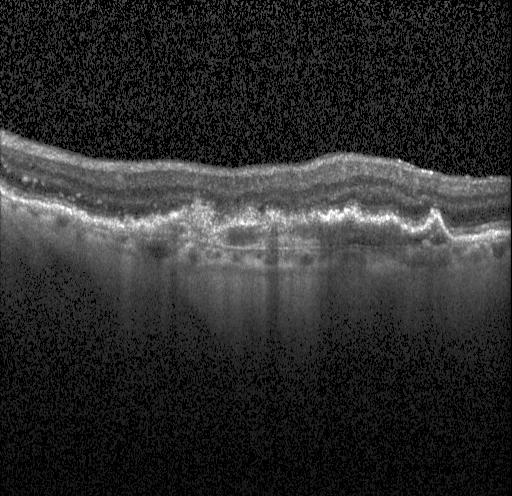
This B-scan demonstrates choroidal neovascularization (CNV).